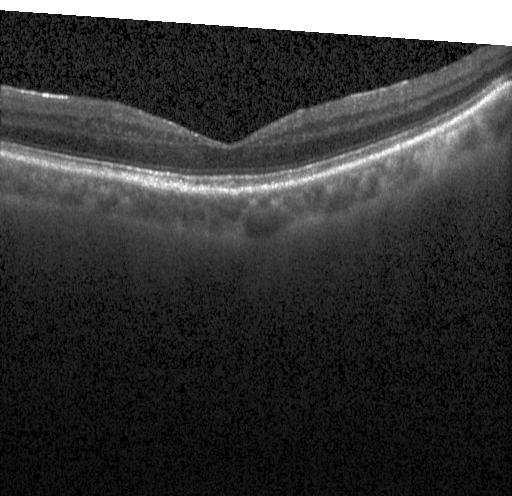

No CNV, no DME, and no drusen.